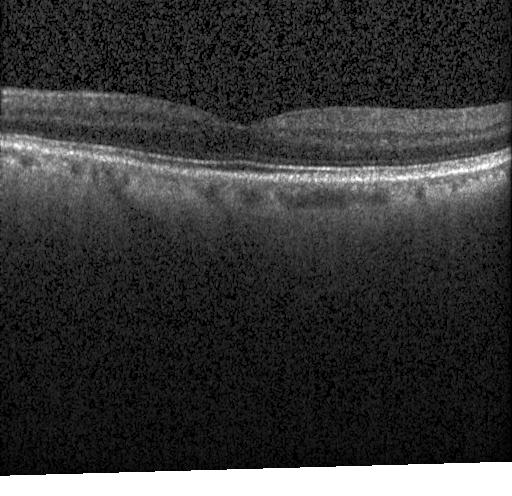

OCT line scan
No choroidal neovascularization, diabetic macular edema, or drusen.